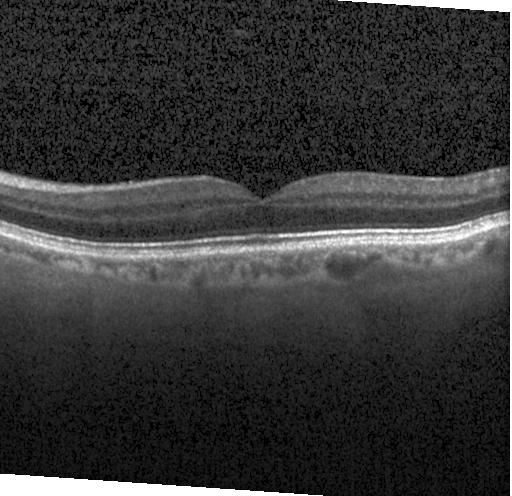

Optical coherence tomography scan. Fovea-centered. SD-OCT. Heidelberg Spectralis.
Assessment: neither CNV, DME, nor drusen.